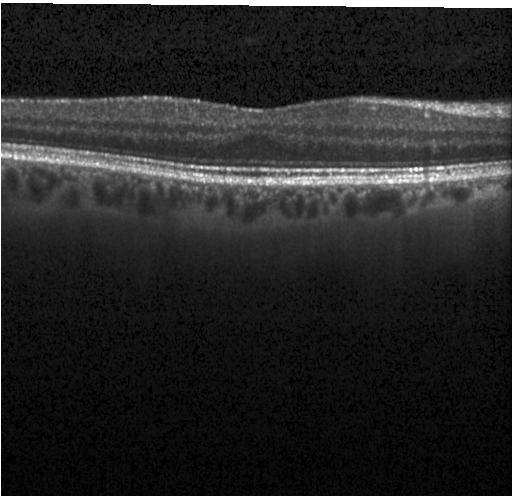 SD-OCT; OCT B-scan; fovea-centered — Macular OCT: neither CNV, DME, nor drusen.